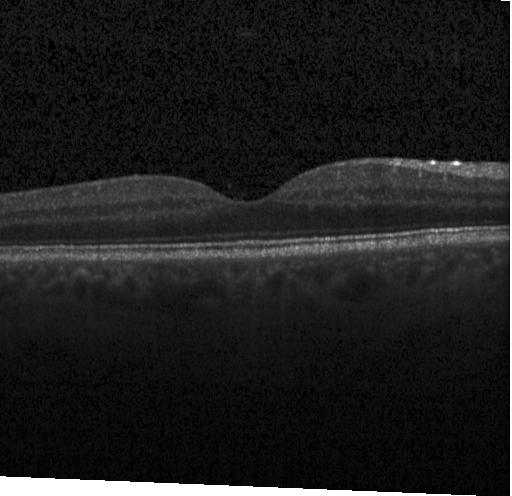 Optical coherence tomography B-scan
The scan shows no choroidal neovascularization, diabetic macular edema, or drusen.